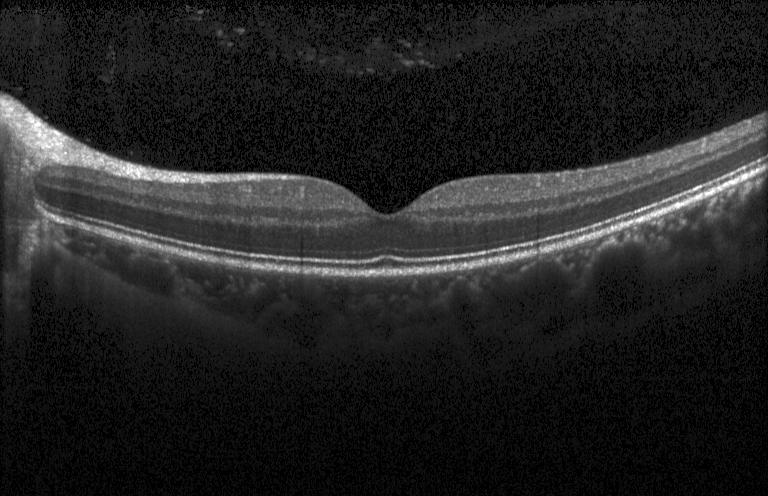 Diagnosis: neither choroidal neovascularization, diabetic macular edema, nor drusen.